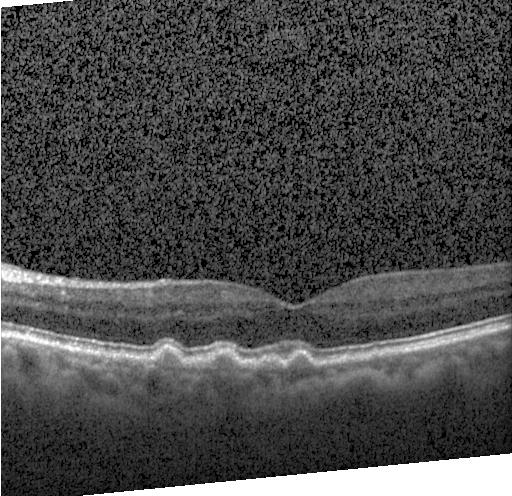
Impression: sub-RPE drusenoid deposits.